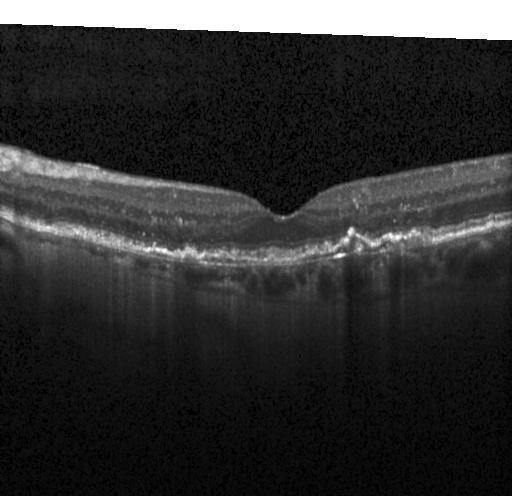 OCT line scan · spectral-domain optical coherence tomography · through the macula. Assessment: drusen.